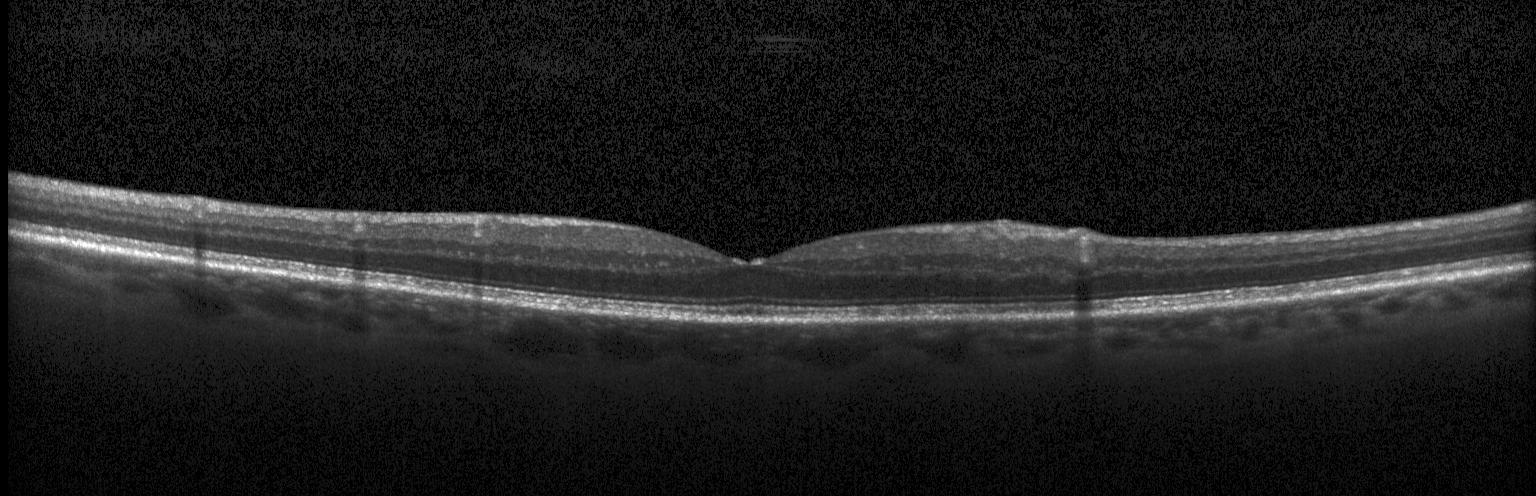

Impression: neither choroidal neovascularization, diabetic macular edema, nor drusen.